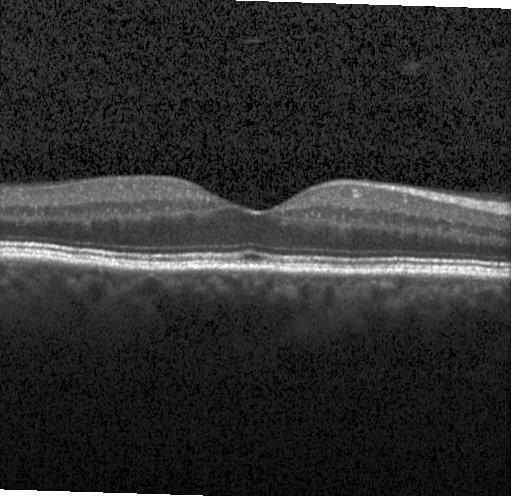 Diagnosis: no CNV, DME, or drusen.